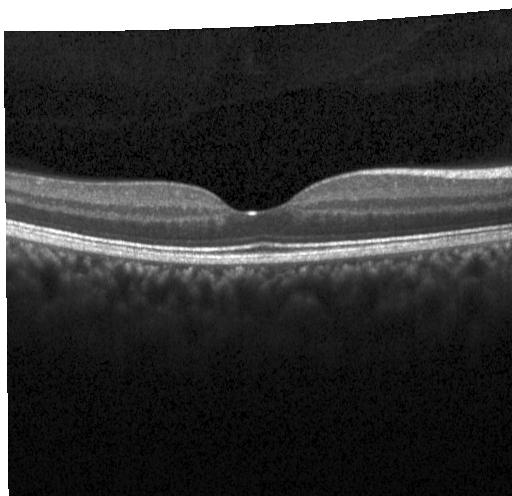
Dx: no CNV, no DME, and no drusen.